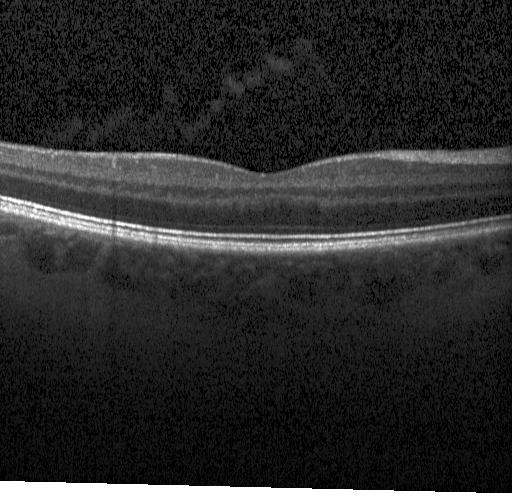 SD-OCT, retinal OCT B-scan.
Assessment: neither CNV, DME, nor drusen.